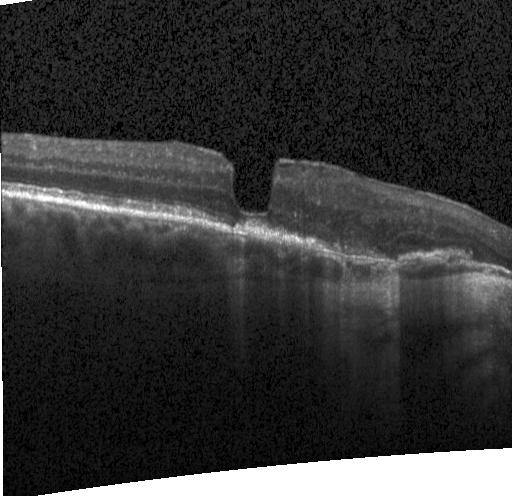
OCT B-scan
Diagnosis: choroidal neovascularization.